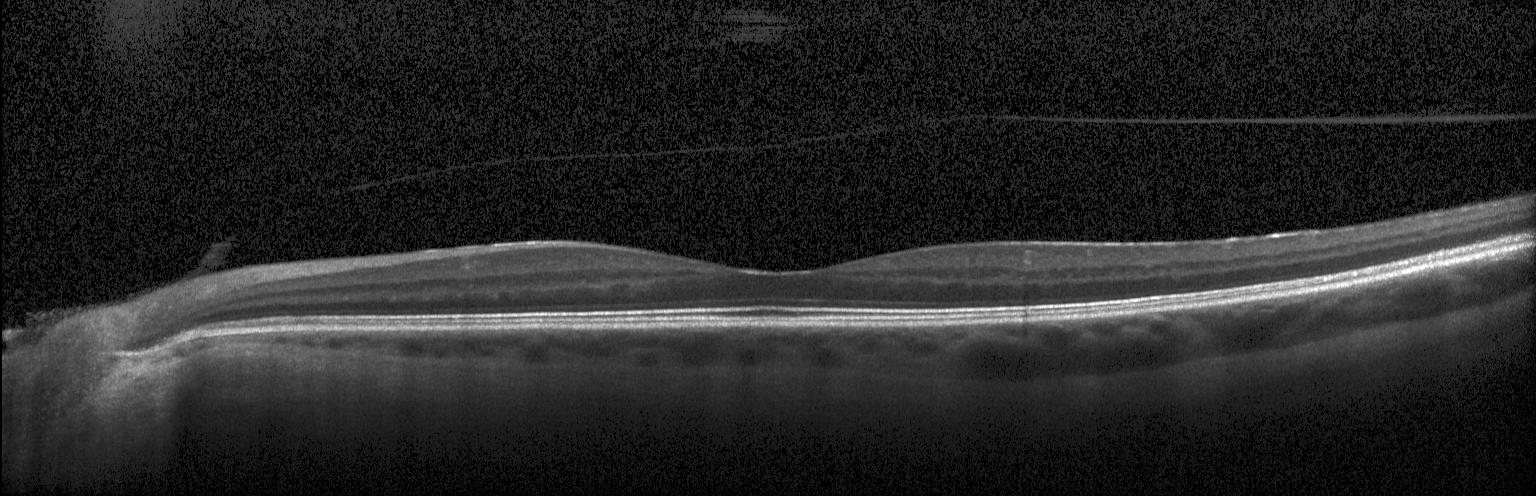 Fovea-centered; instrument: Heidelberg Spectralis; spectral-domain OCT; optical coherence tomography scan.
No evidence of CNV, DME, or drusen.